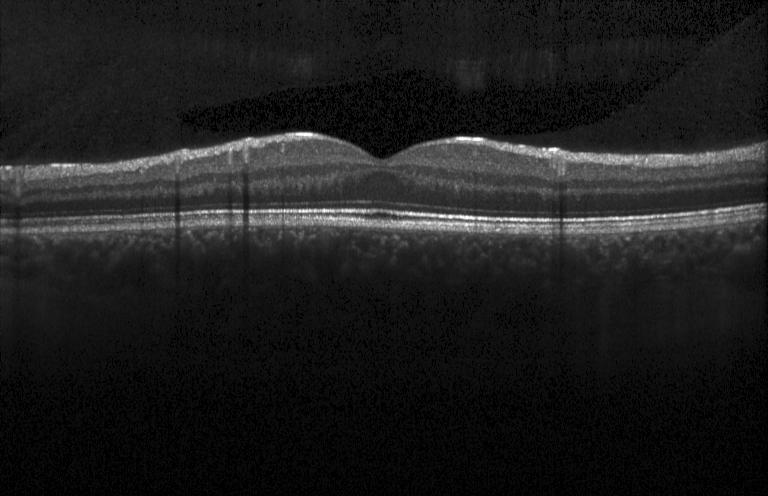 Impression: no choroidal neovascularization, diabetic macular edema, or drusen.